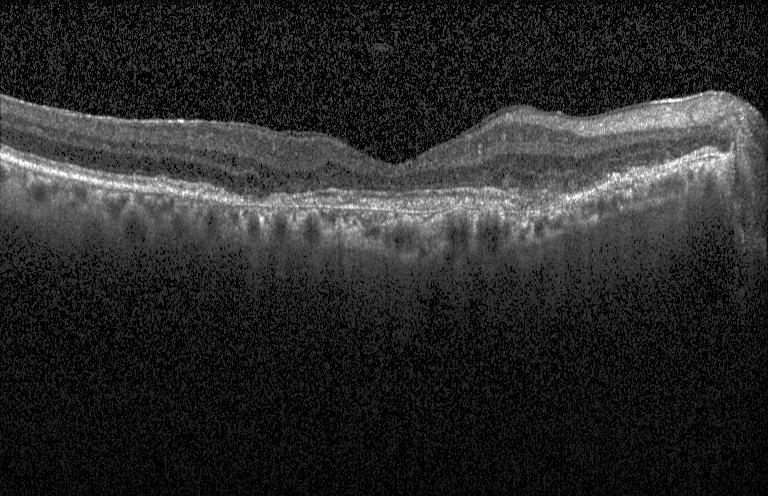
Heidelberg Spectralis. Spectral-domain OCT. Optical coherence tomography B-scan. Fovea-centered. Diagnosis: choroidal neovascularization (CNV).